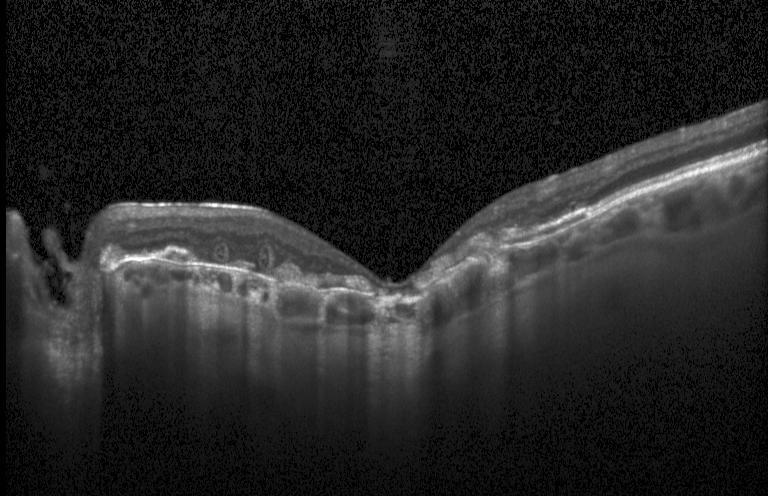

Horizontal scan through the fovea; spectral-domain OCT; OCT B-scan
This B-scan demonstrates CNV.